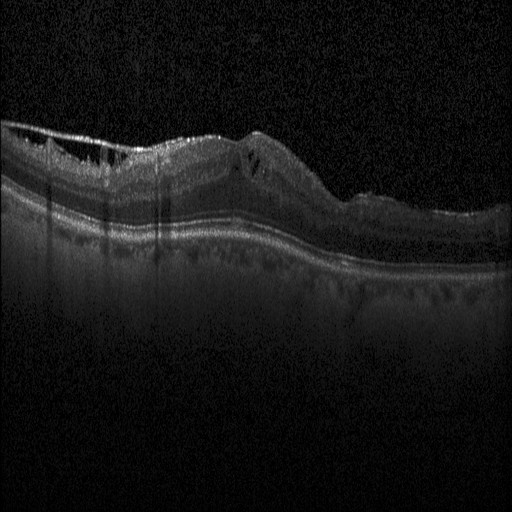
Assessment: DME.